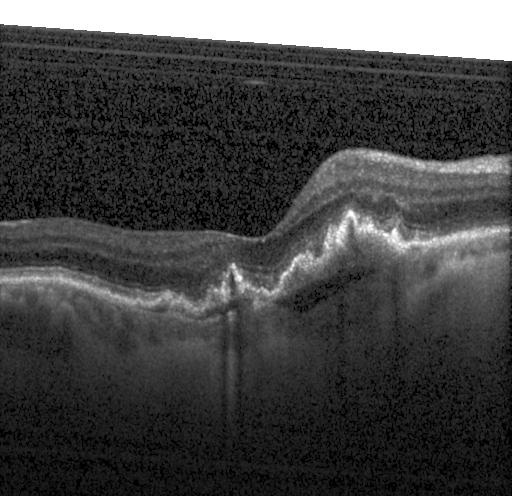
Through the macula. Optical coherence tomography B-scan. Instrument: Heidelberg Spectralis. Dx: choroidal neovascularization.